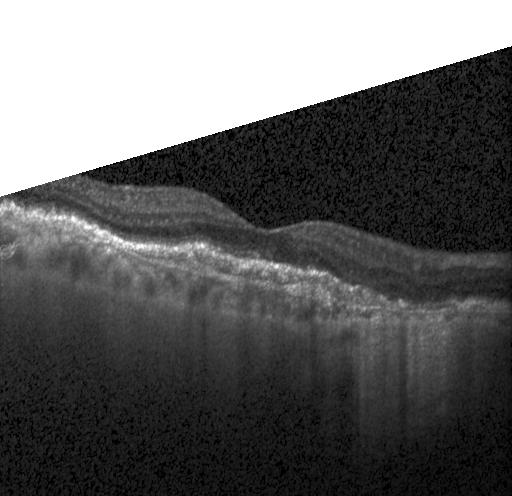 Retinal OCT cross-section, acquired on a Heidelberg Spectralis, SD-OCT — This B-scan demonstrates a choroidal neovascular membrane.